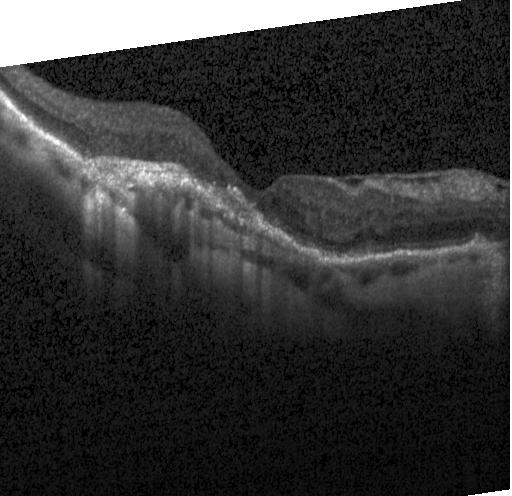
OCT finding: CNV.